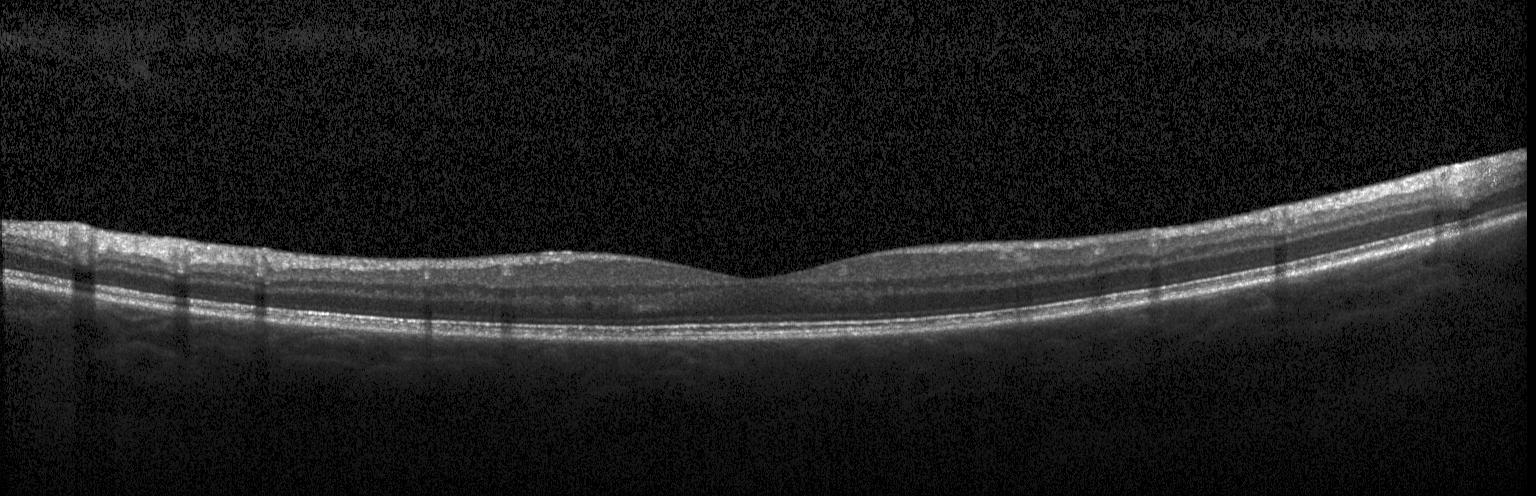
OCT scan showing no choroidal neovascularization, no diabetic macular edema, and no drusen.